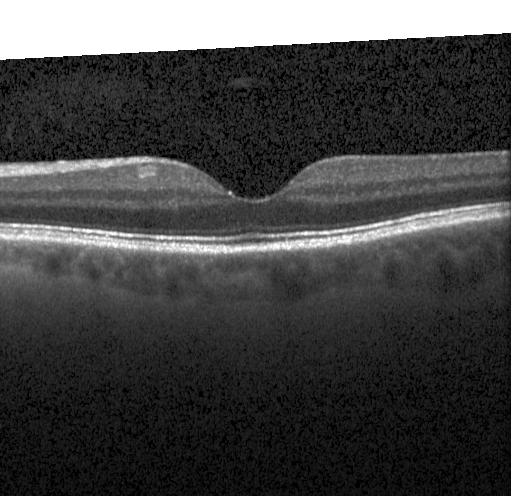 Retinal OCT cross-section. Assessment: no evidence of choroidal neovascularization, diabetic macular edema, or drusen.